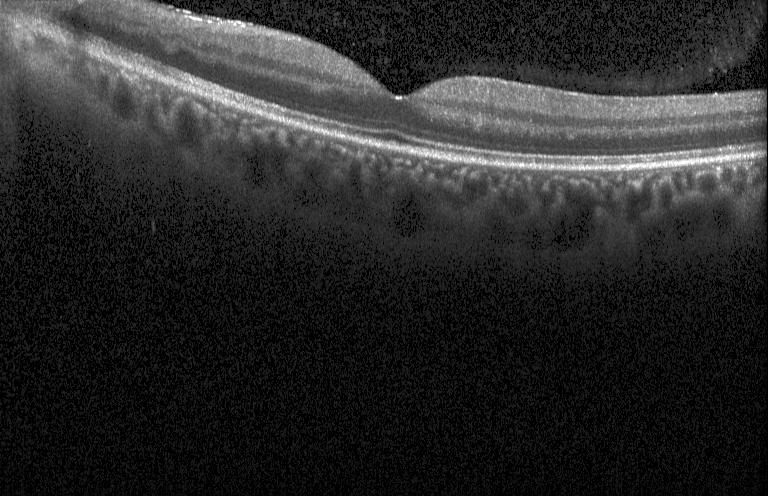 Optical coherence tomography scan. Spectral-domain OCT. Heidelberg Spectralis OCT system. Finding: no choroidal neovascularization, diabetic macular edema, or drusen.